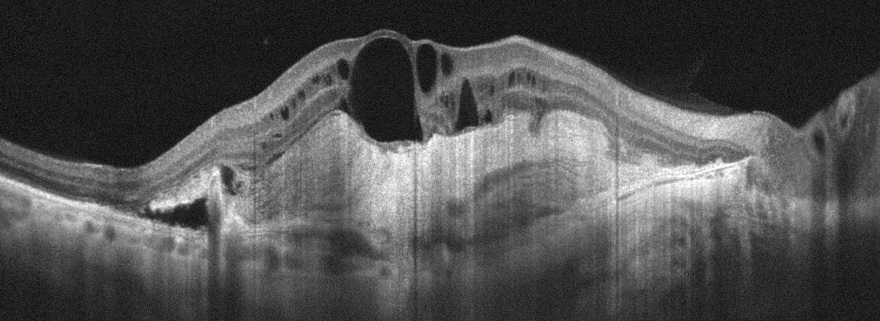
OCT line scan. Diagnosis: age-related macular degeneration.